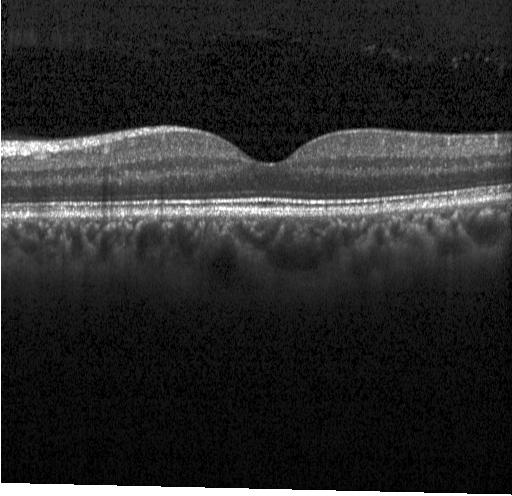

Optical coherence tomography scan — The scan shows no CNV, DME, or drusen.